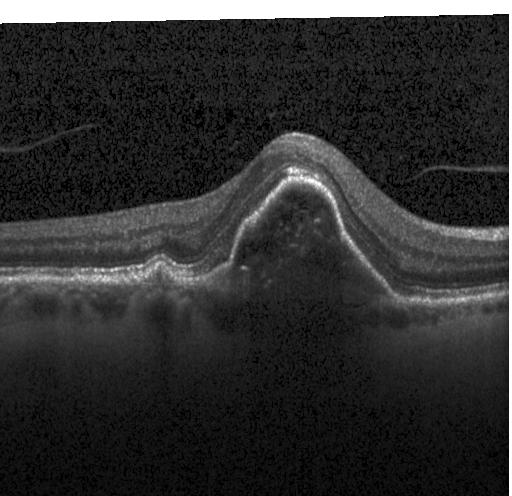

Diagnosis: choroidal neovascularization.